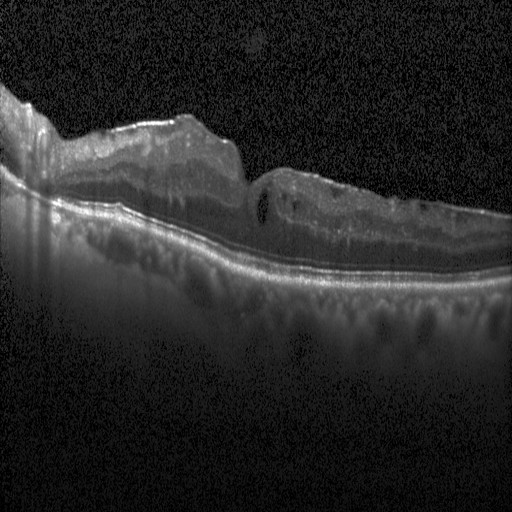
This B-scan demonstrates DME.